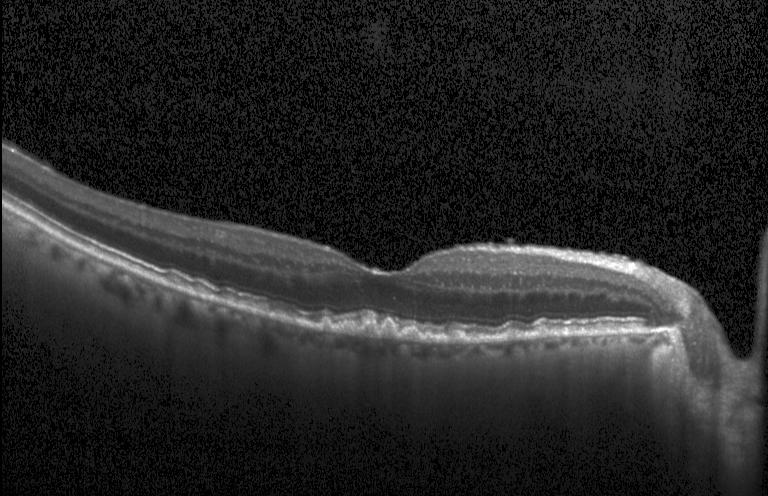 Retinal OCT B-scan; spectral-domain optical coherence tomography; fovea-centered. Diagnosis: multiple drusen.